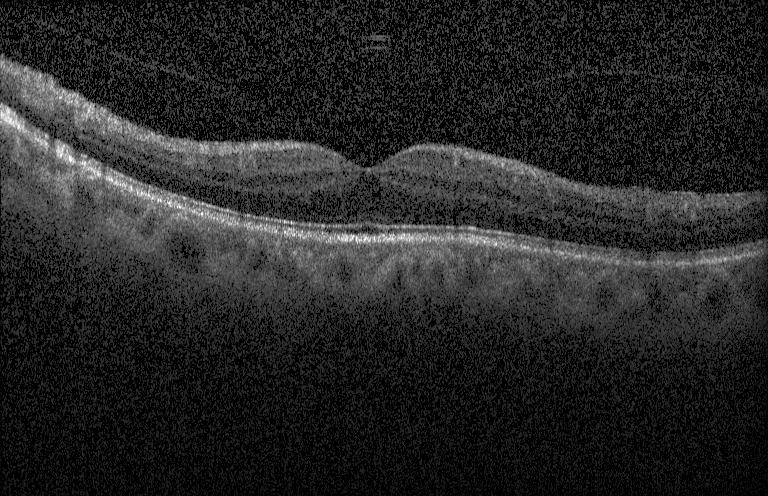 Optical coherence tomography B-scan.
OCT finding: no evidence of CNV, DME, or drusen.